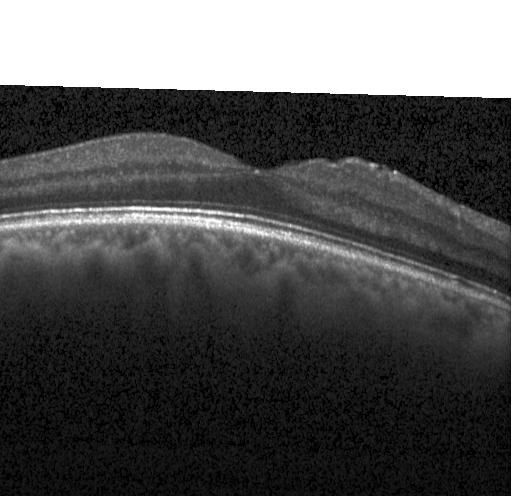

Finding: no CNV, no DME, and no drusen.